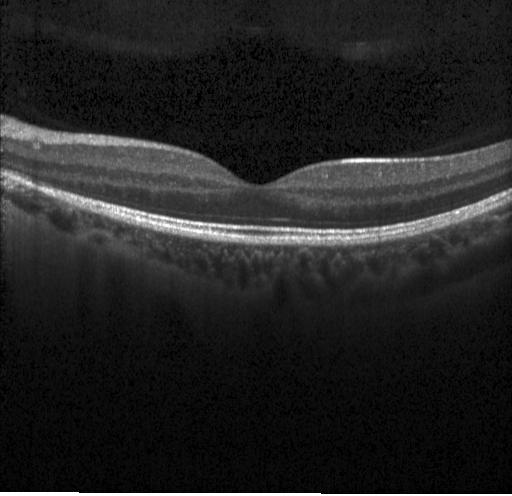
Optical coherence tomography B-scan. Assessment: no choroidal neovascularization, no diabetic macular edema, and no drusen.